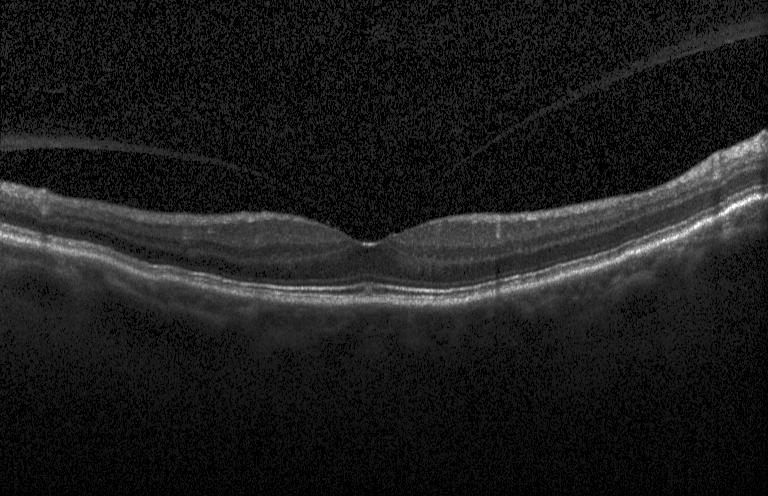 Heidelberg Spectralis OCT system, OCT B-scan, through the macula, spectral-domain OCT
Finding: no choroidal neovascularization, diabetic macular edema, or drusen.